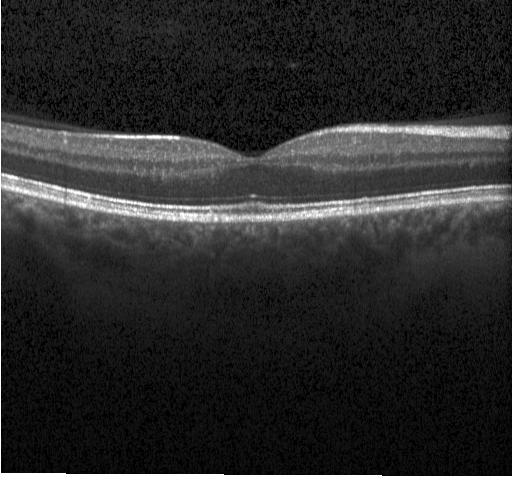
OCT B-scan
Macular OCT: no choroidal neovascularization, no diabetic macular edema, and no drusen.